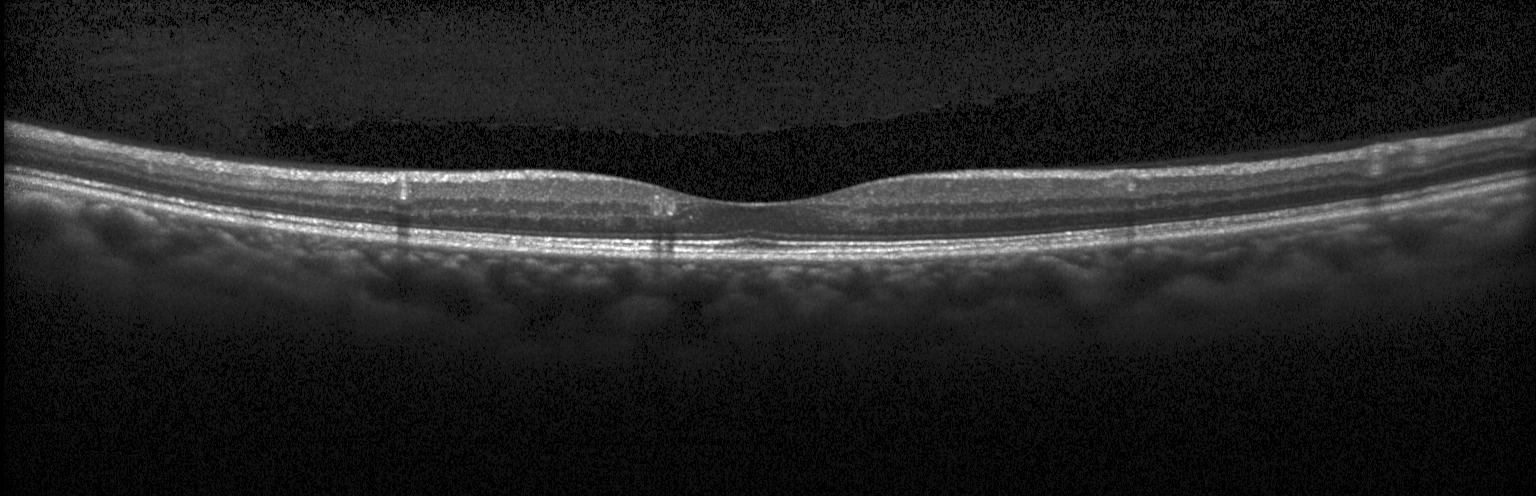

OCT line scan; spectral-domain optical coherence tomography
Impression: no CNV, no DME, and no drusen.